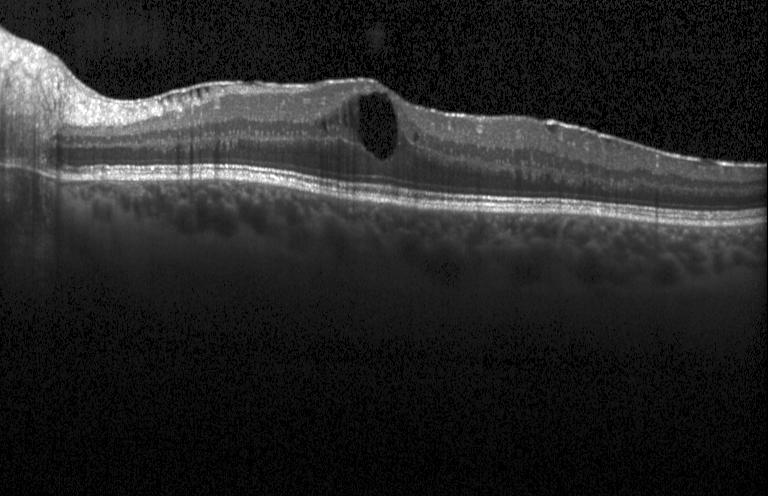

Impression: diabetic macular edema.